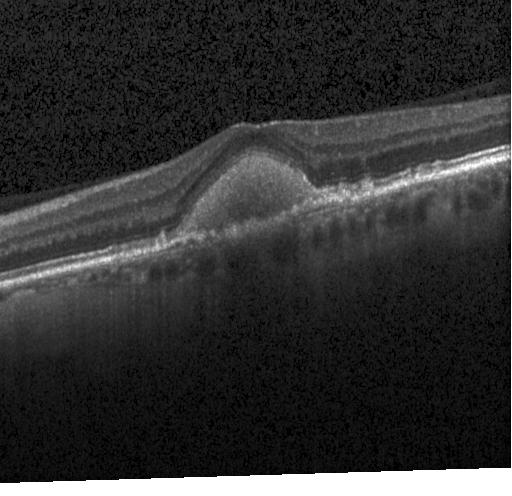 Retinal OCT cross-section. Through the macula. Heidelberg Spectralis
Diagnosis: a choroidal neovascular membrane.